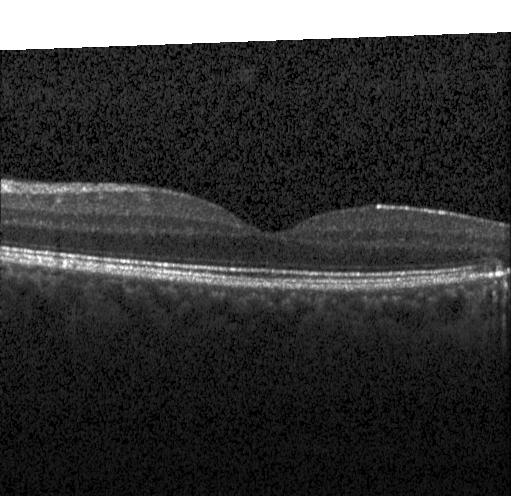 Heidelberg Spectralis, retinal OCT B-scan, centered on the fovea
Dx: no choroidal neovascularization, diabetic macular edema, or drusen.